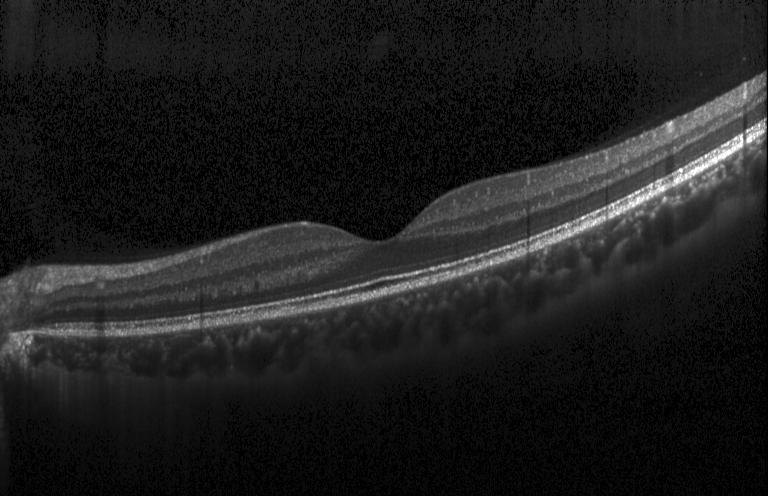 OCT scan showing no choroidal neovascularization, no diabetic macular edema, and no drusen.